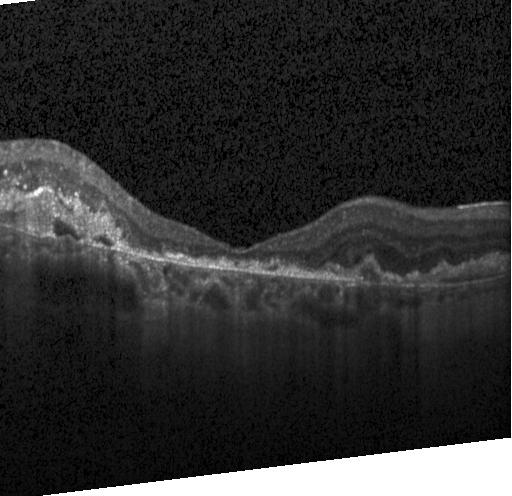

Centered on the fovea. Heidelberg Spectralis. Spectral-domain optical coherence tomography. Optical coherence tomography scan. The scan shows a choroidal neovascular membrane.